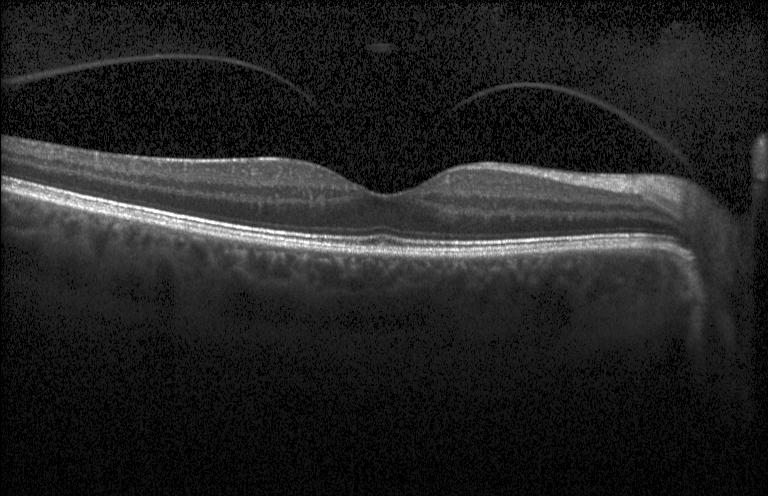
Impression: neither choroidal neovascularization, diabetic macular edema, nor drusen.